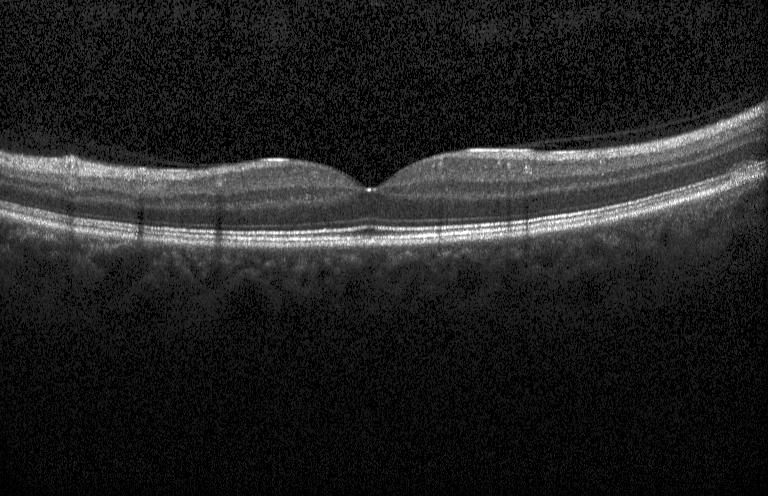
Optical coherence tomography B-scan, fovea-centered, acquired on a Heidelberg Spectralis. Finding: no choroidal neovascularization, diabetic macular edema, or drusen.